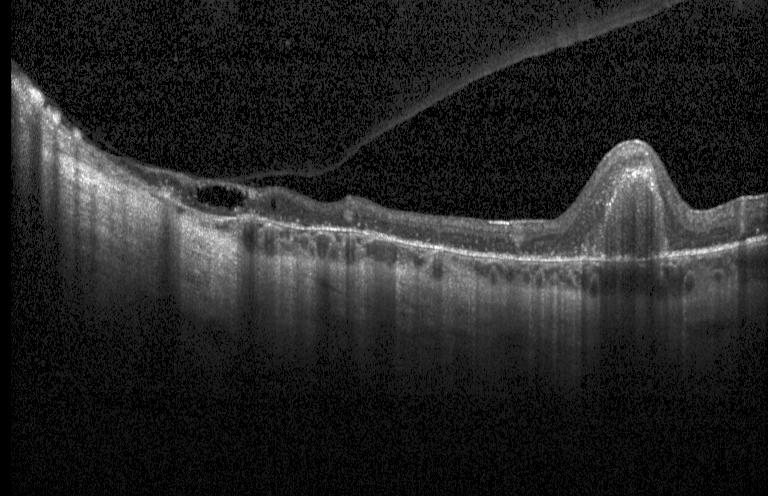
Finding: a choroidal neovascular membrane.